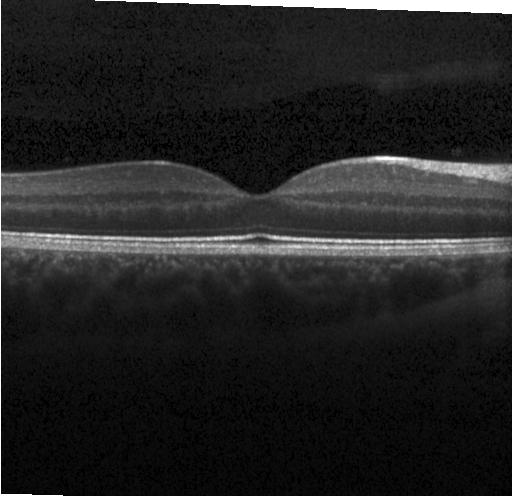
SD-OCT, optical coherence tomography B-scan, acquired on a Heidelberg Spectralis, fovea-centered — This B-scan demonstrates no choroidal neovascularization, no diabetic macular edema, and no drusen.